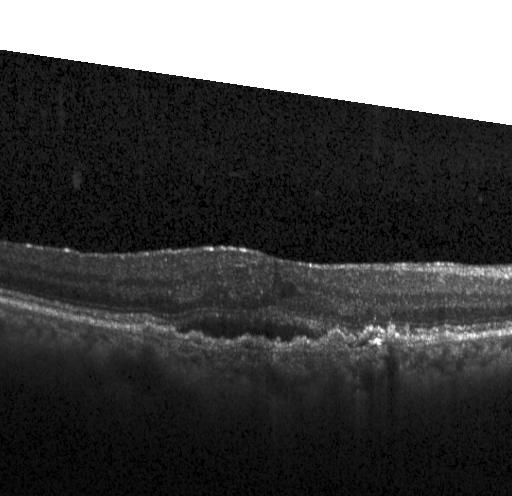
Optical coherence tomography scan.
A choroidal neovascular membrane.